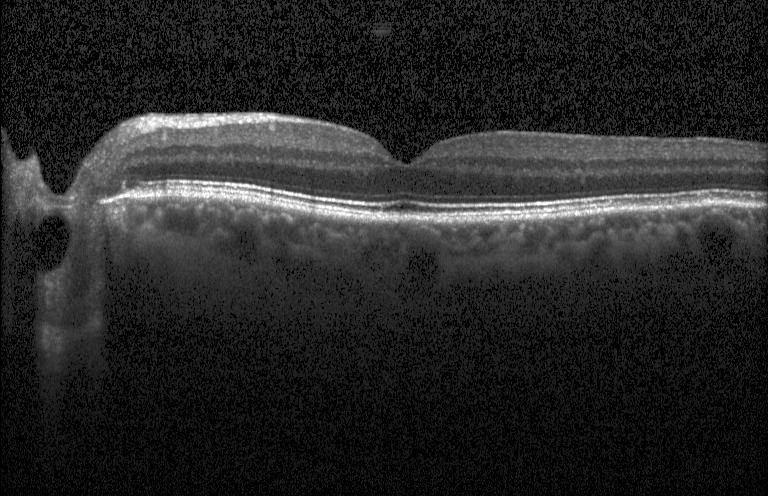 Fovea-centered · retinal OCT cross-section · Heidelberg Spectralis OCT system · spectral-domain OCT — Finding: no CNV, no DME, and no drusen.